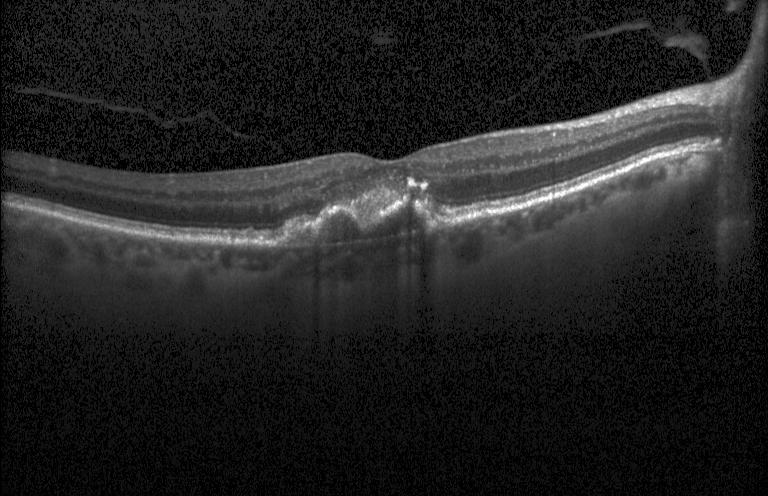

Retinal OCT cross-section · fovea-centered. Macular OCT: choroidal neovascularization (CNV).